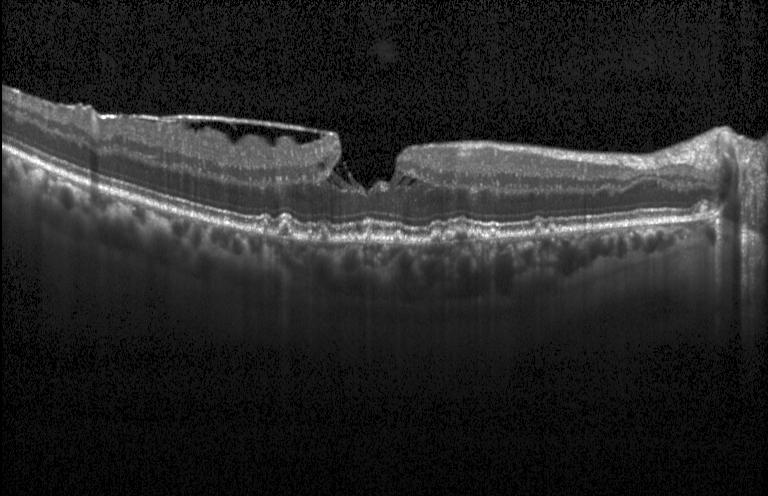
OCT B-scan.
Assessment: drusen.